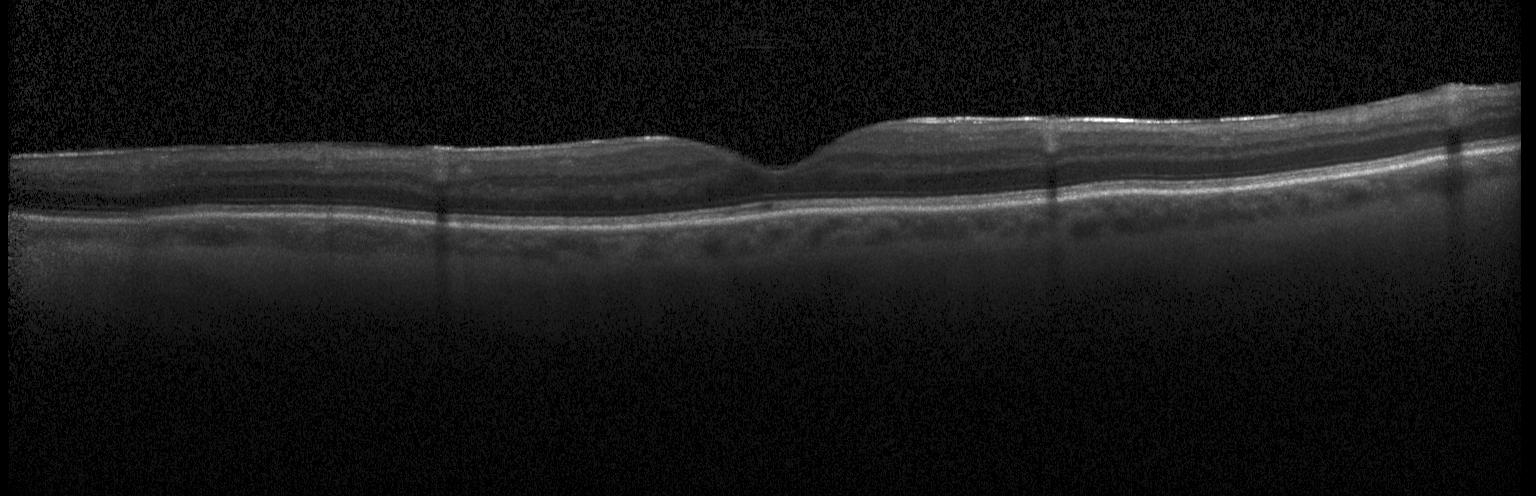
Spectral-domain OCT; Heidelberg Spectralis; centered on the fovea; optical coherence tomography scan — OCT finding: no choroidal neovascularization, diabetic macular edema, or drusen.